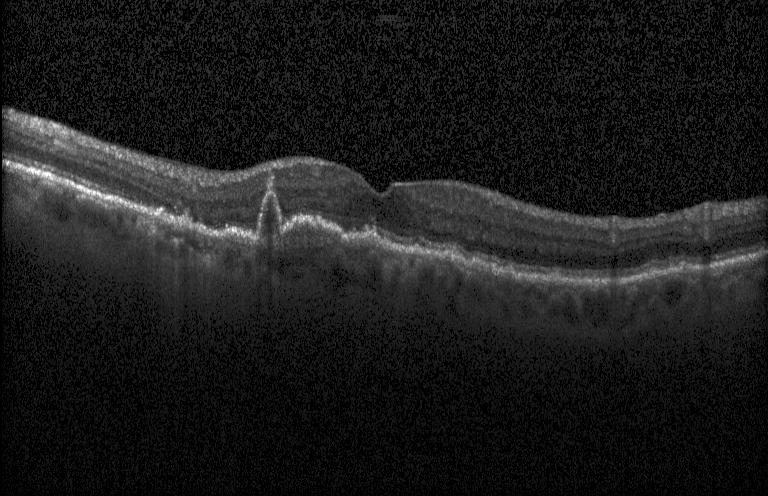
OCT finding: a choroidal neovascular membrane.